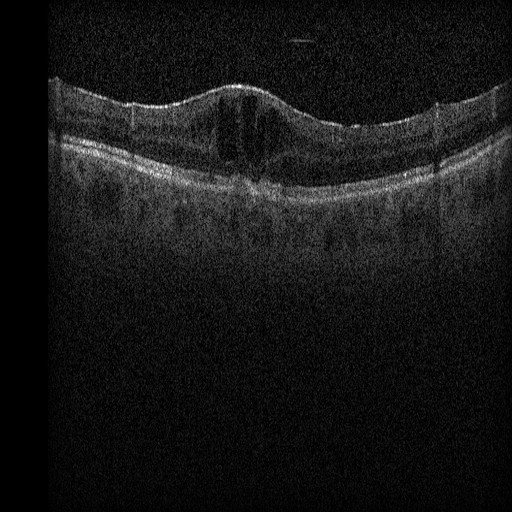
Optical coherence tomography scan · horizontal scan through the fovea. OCT finding: DME.